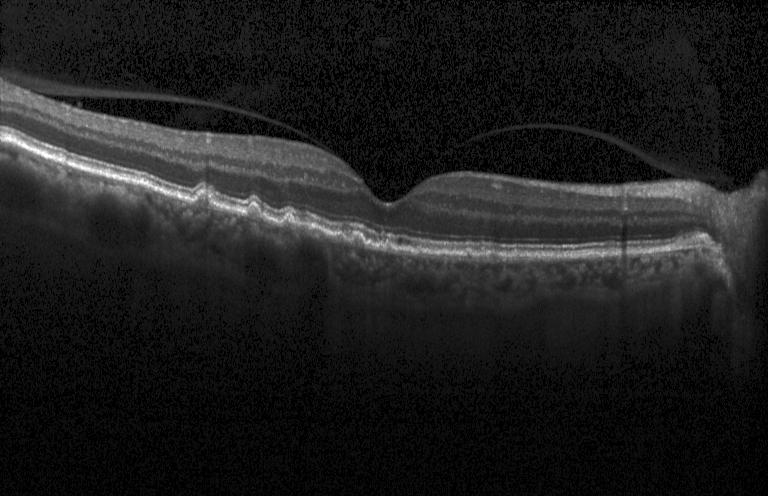 Heidelberg Spectralis. SD-OCT. Horizontal scan through the fovea. OCT B-scan. Diagnosis: multiple drusen.